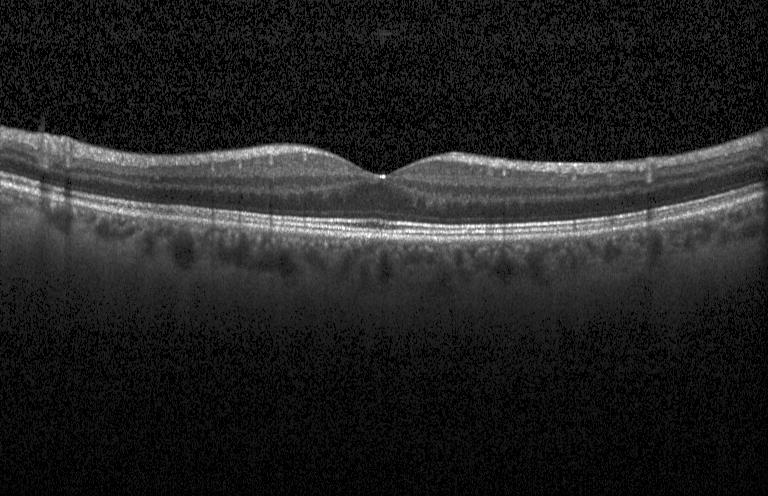

Acquired on a Heidelberg Spectralis. Through the macula. SD-OCT. OCT B-scan
Finding: neither CNV, DME, nor drusen.